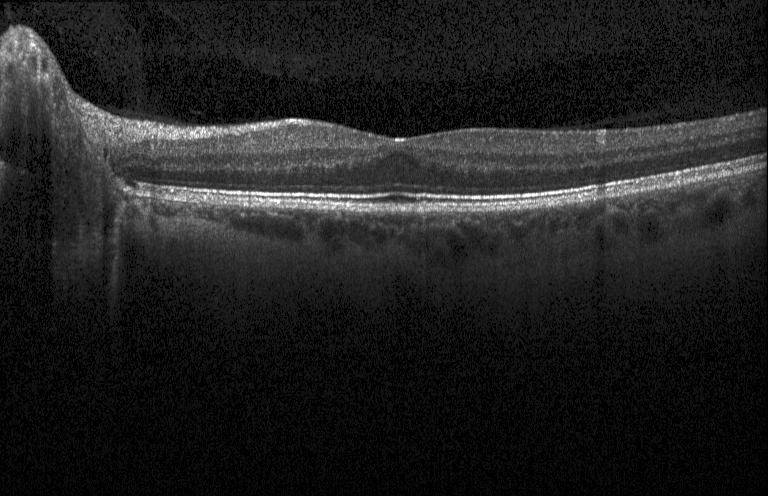 Retinal OCT B-scan · Heidelberg Spectralis OCT system. Impression: no evidence of choroidal neovascularization, diabetic macular edema, or drusen.